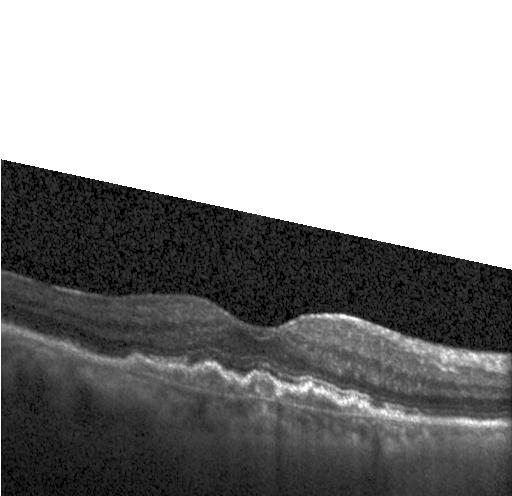
Fovea-centered. SD-OCT. Optical coherence tomography scan. Instrument: Heidelberg Spectralis — Finding: a choroidal neovascular membrane.